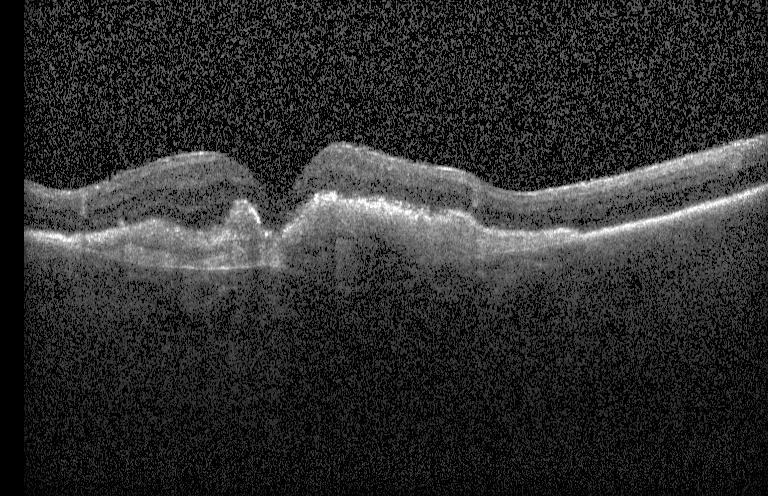

Macular OCT: CNV.